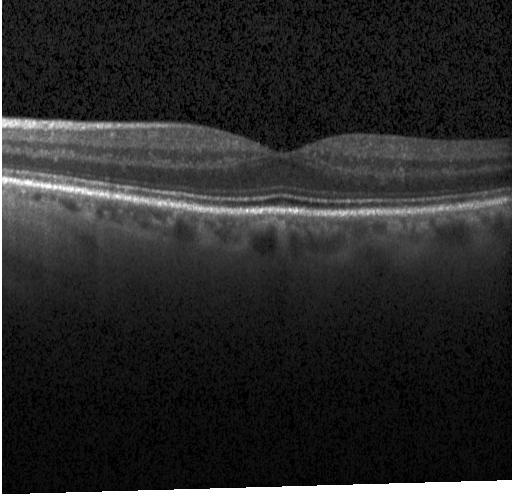

Instrument: Heidelberg Spectralis · OCT line scan.
This B-scan demonstrates no CNV, DME, or drusen.